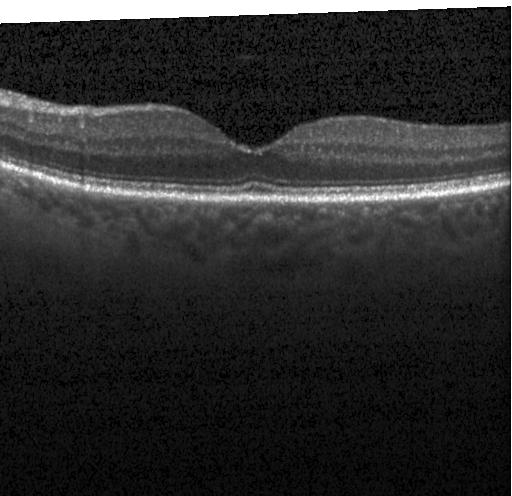 Macular OCT demonstrating no choroidal neovascularization, diabetic macular edema, or drusen.